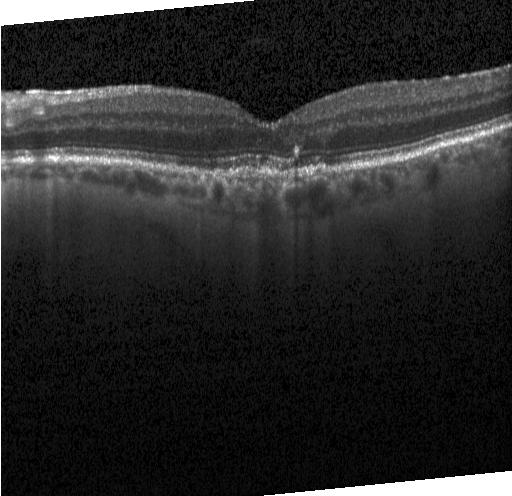
OCT finding: a choroidal neovascular membrane.